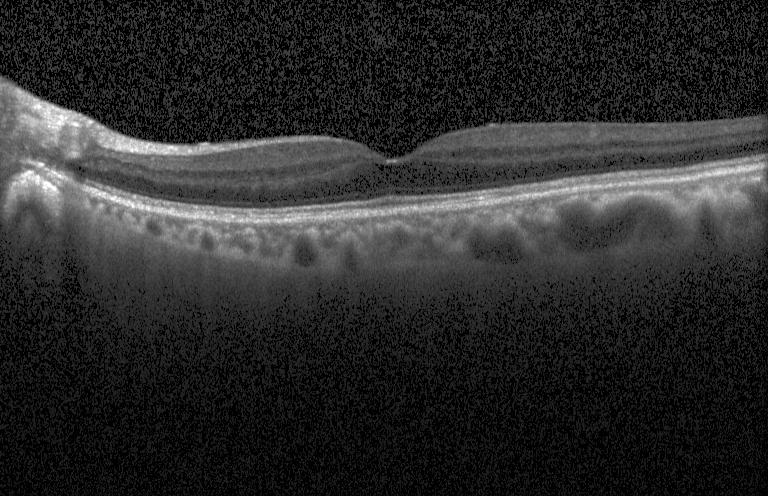 Macular OCT demonstrating no choroidal neovascularization, no diabetic macular edema, and no drusen.